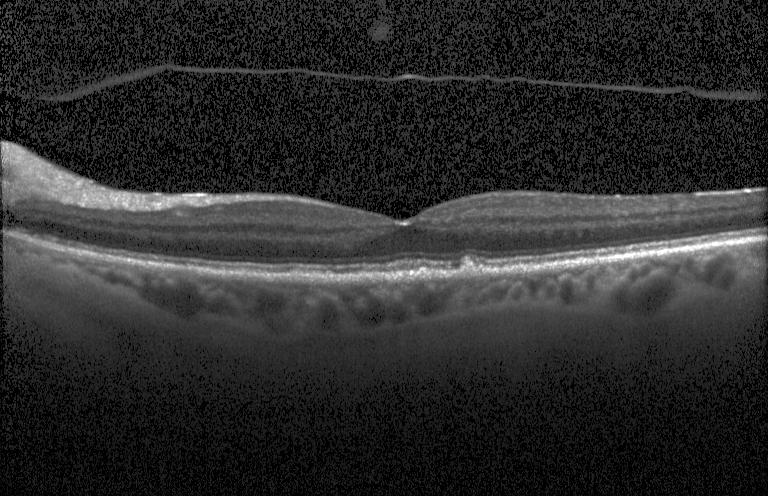
Dx: multiple drusen.